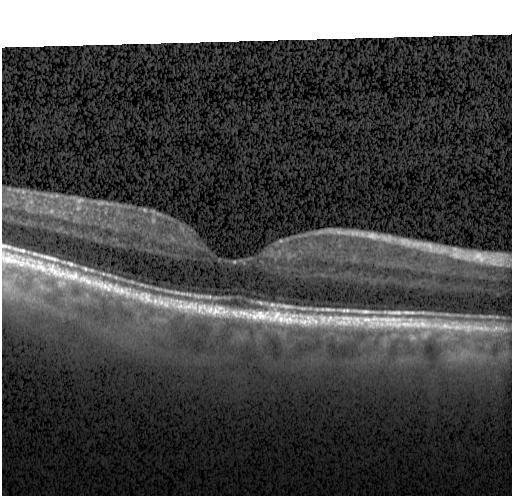

OCT B-scan.
This B-scan demonstrates no choroidal neovascularization, diabetic macular edema, or drusen.